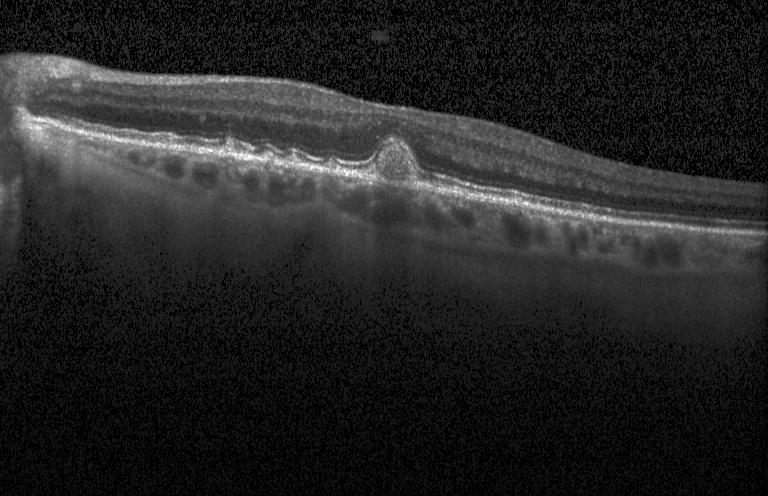
Fovea-centered. SD-OCT. OCT B-scan. Instrument: Heidelberg Spectralis.
Dx: choroidal neovascularization.